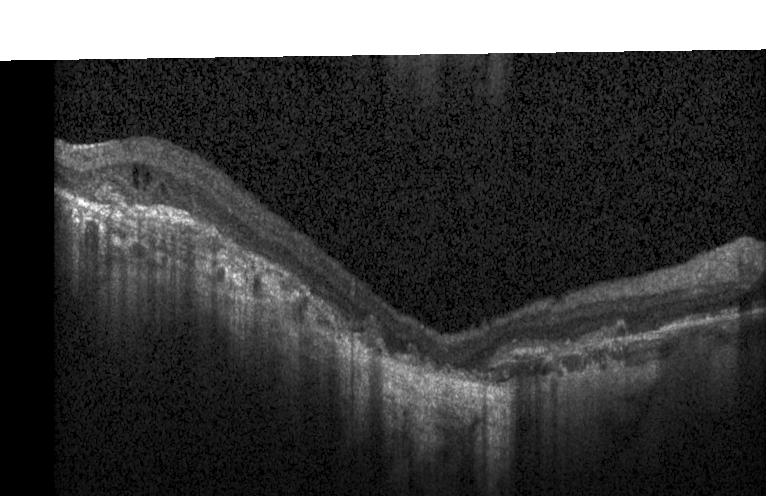

Diagnosis: a choroidal neovascular membrane.